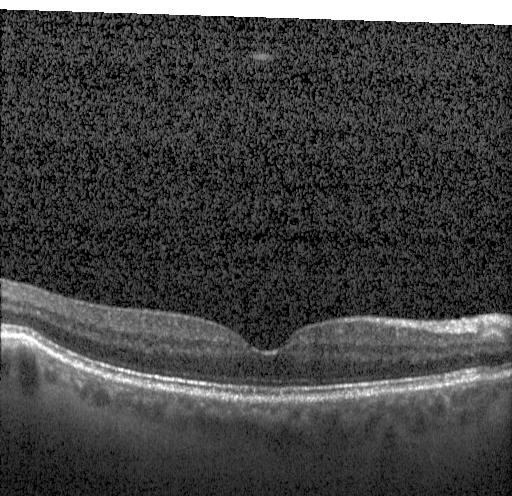 Spectral-domain OCT; horizontal scan through the fovea; optical coherence tomography scan; Heidelberg Spectralis OCT system.
OCT finding: no choroidal neovascularization, no diabetic macular edema, and no drusen.